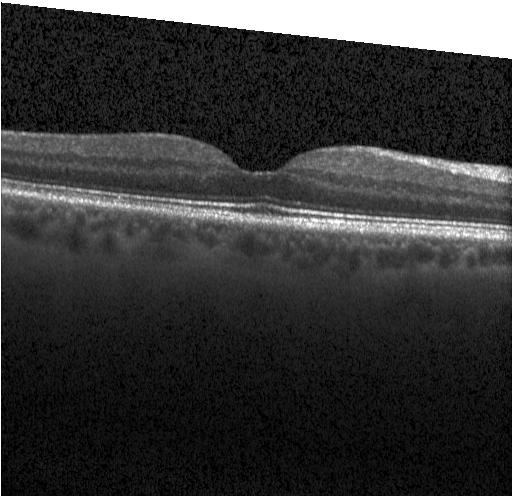
Diagnosis: no choroidal neovascularization, diabetic macular edema, or drusen.